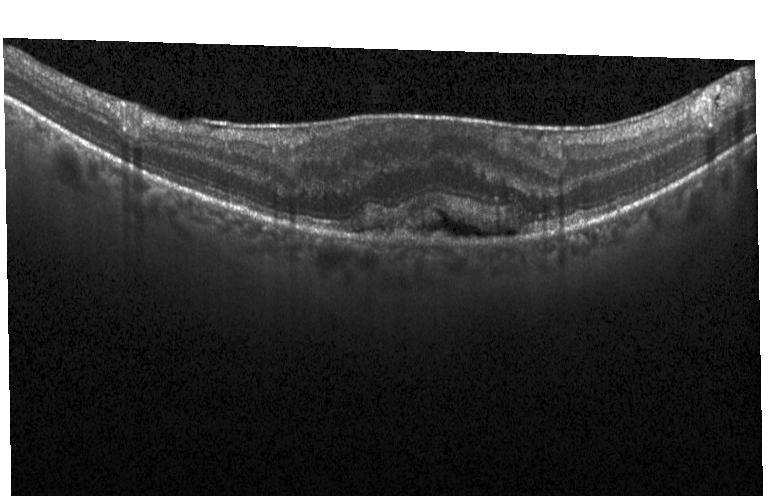 Retinal OCT cross-section; horizontal scan through the fovea.
This B-scan demonstrates choroidal neovascularization.